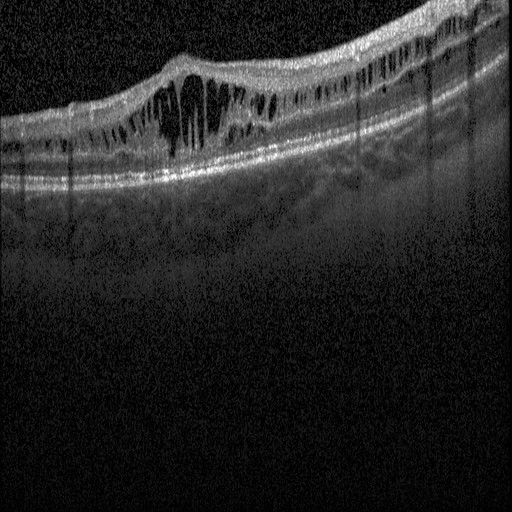 OCT B-scan; macular scan. Diagnosis: diabetic macular edema (DME).